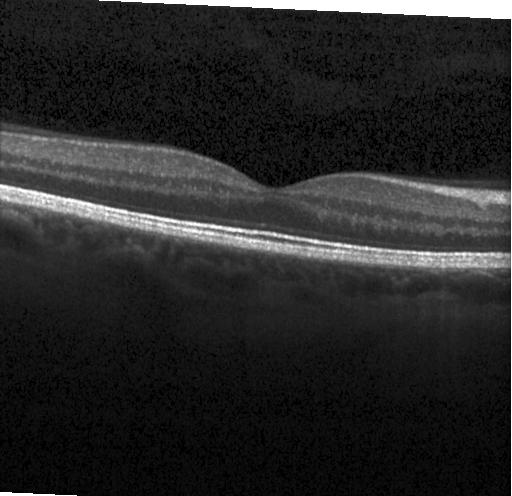 Optical coherence tomography scan.
Assessment: neither choroidal neovascularization, diabetic macular edema, nor drusen.